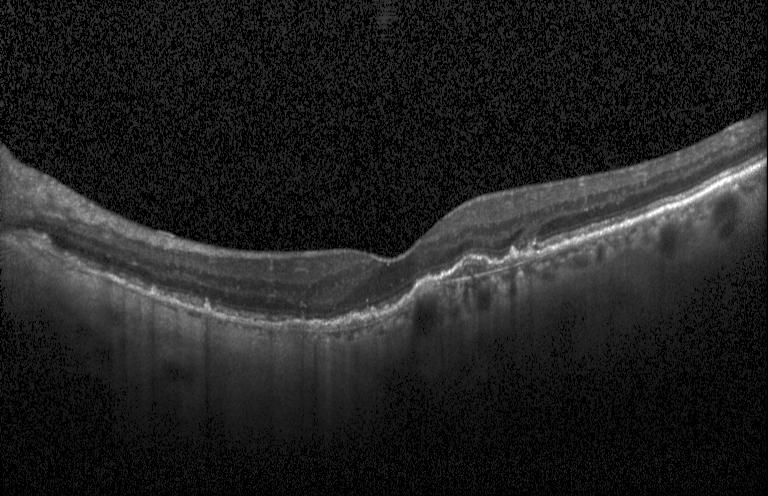 Instrument: Heidelberg Spectralis. OCT B-scan. Horizontal scan through the fovea. Spectral-domain OCT
This B-scan demonstrates choroidal neovascularization.